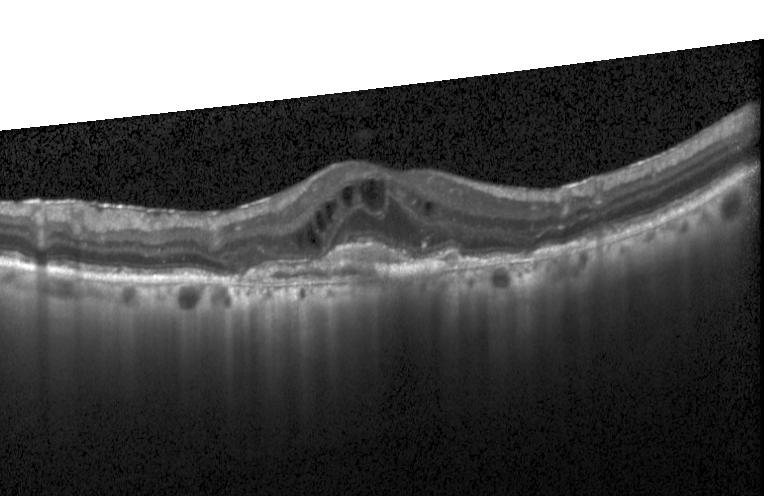

Heidelberg Spectralis, retinal OCT cross-section, macular scan — Assessment: choroidal neovascularization.